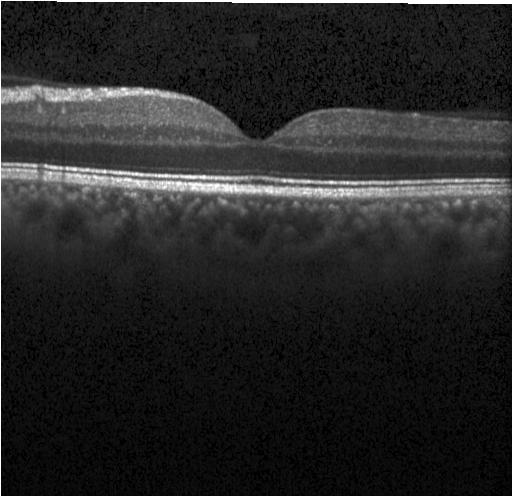

Retinal OCT cross-section — Finding: no evidence of choroidal neovascularization, diabetic macular edema, or drusen.